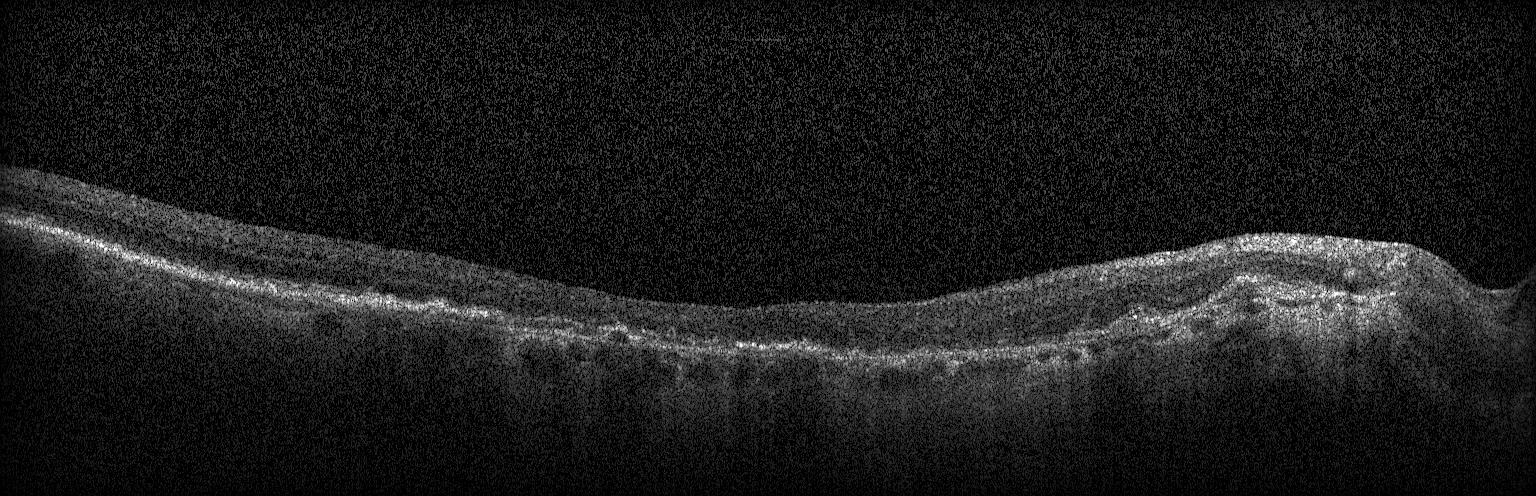

This B-scan demonstrates a choroidal neovascular membrane.